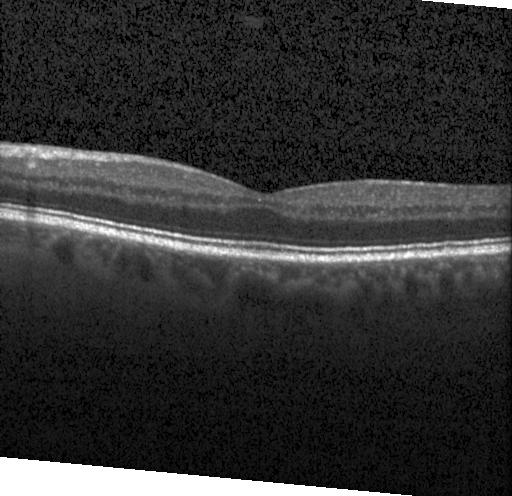 Acquired on a Heidelberg Spectralis. Centered on the fovea. Spectral-domain optical coherence tomography. OCT line scan.
Finding: no evidence of CNV, DME, or drusen.